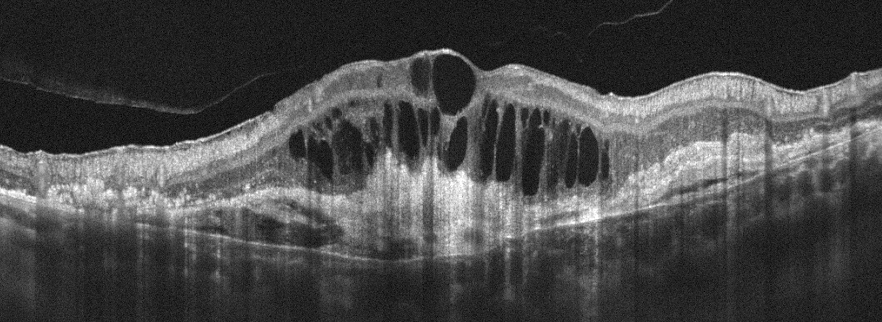

Optical coherence tomography B-scan · left eye. Diagnosis: age-related macular degeneration.